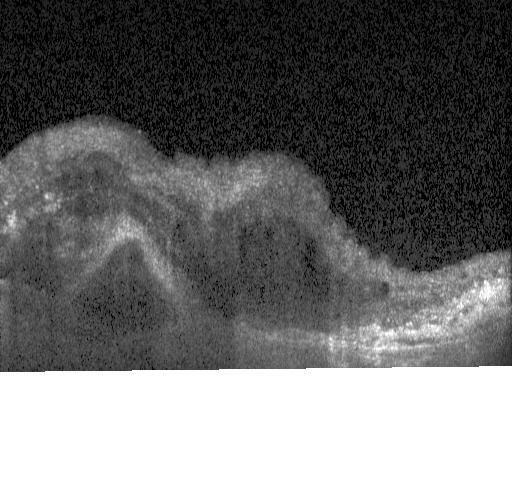 CNV.